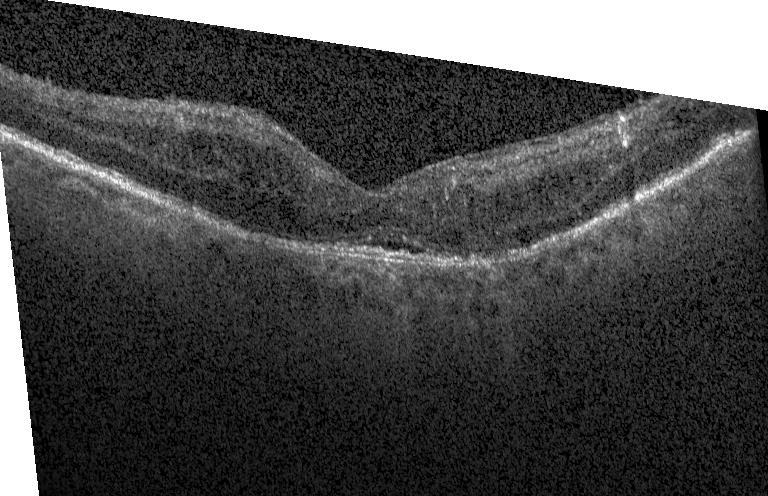
Retinal OCT cross-section — This B-scan demonstrates CNV.